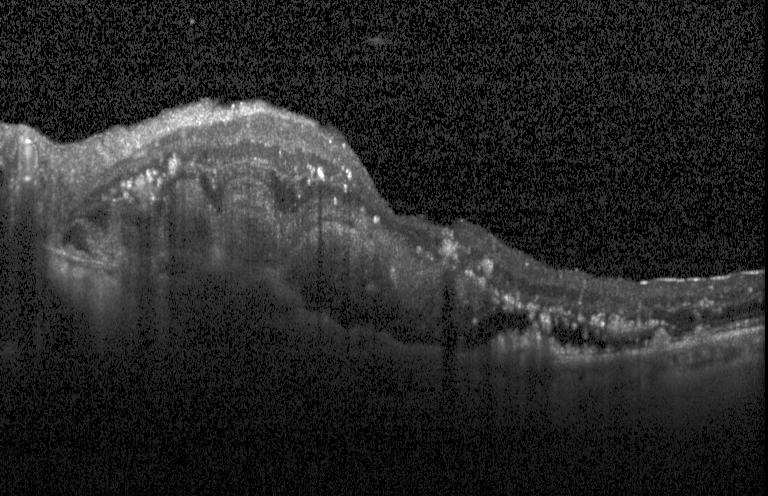
OCT finding: a choroidal neovascular membrane.